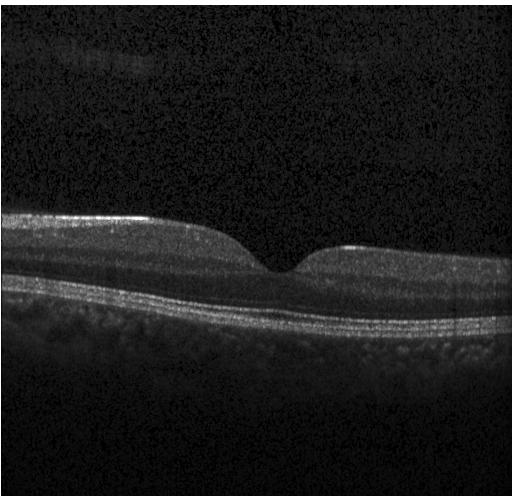

Finding: no choroidal neovascularization, diabetic macular edema, or drusen.